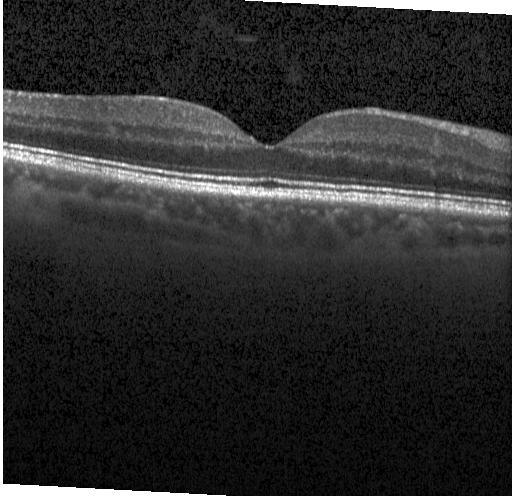 SD-OCT. OCT B-scan — Finding: no evidence of CNV, DME, or drusen.